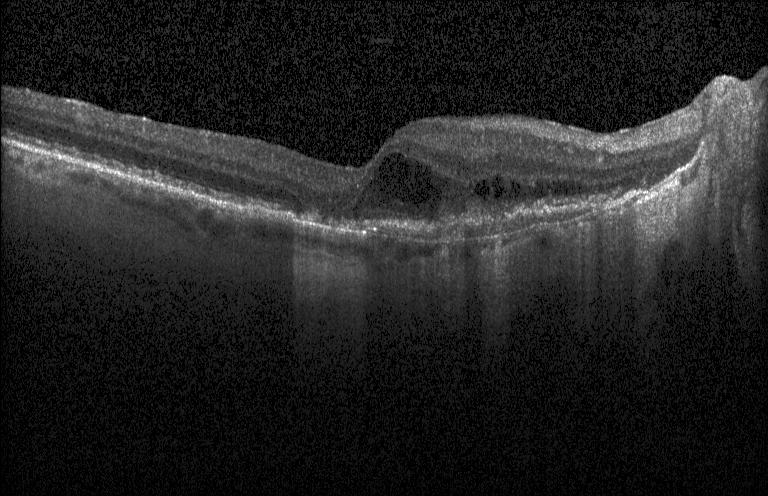 OCT line scan; horizontal scan through the fovea; Heidelberg Spectralis — Impression: a choroidal neovascular membrane.